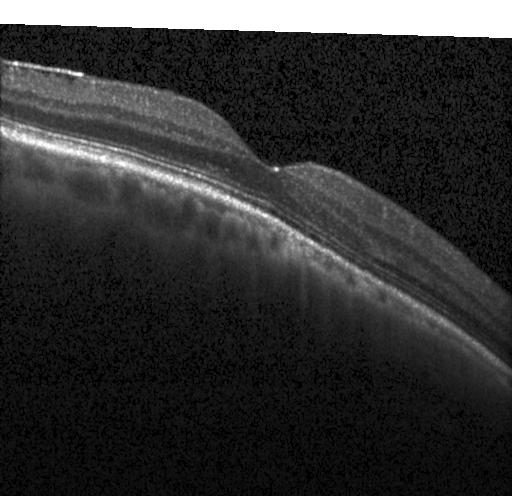
Heidelberg Spectralis. OCT B-scan
Diagnosis: no CNV, no DME, and no drusen.